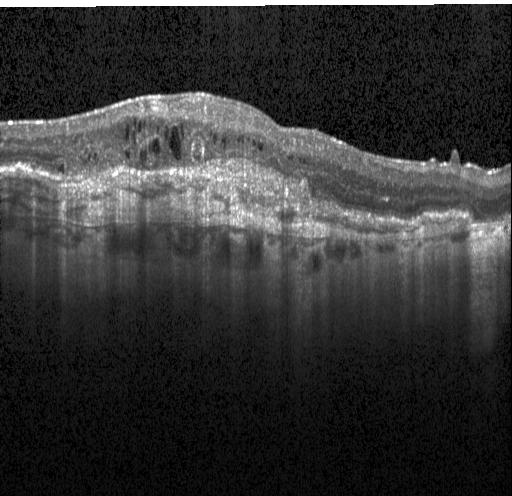
Finding: a choroidal neovascular membrane.